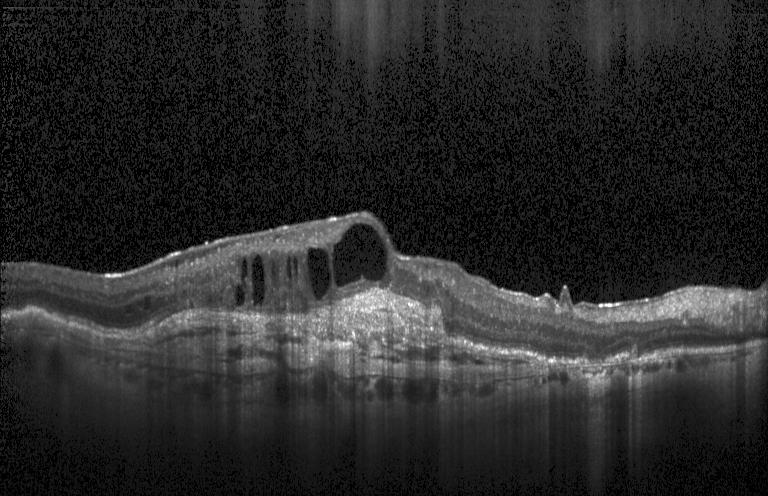

Optical coherence tomography scan; centered on the fovea; spectral-domain optical coherence tomography — Dx: a choroidal neovascular membrane.